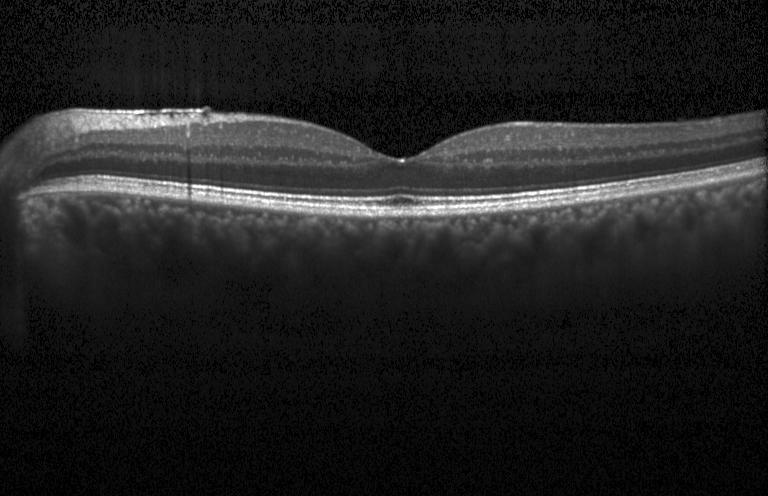
OCT B-scan, Heidelberg Spectralis, spectral-domain optical coherence tomography, macular scan.
Diagnosis: neither choroidal neovascularization, diabetic macular edema, nor drusen.